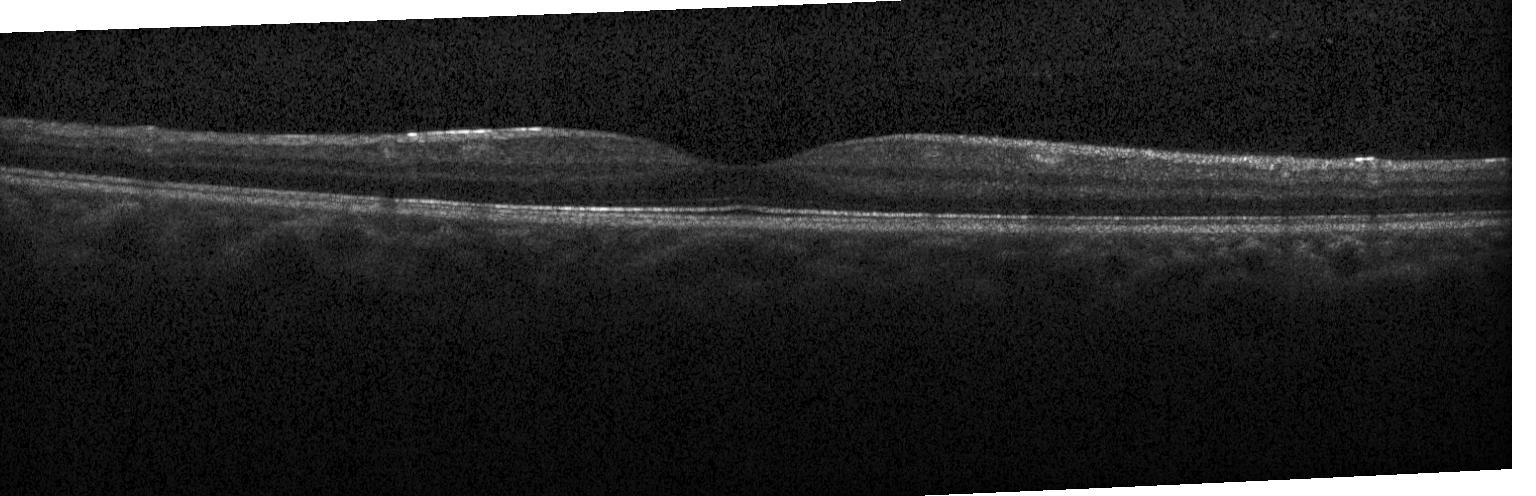
Retinal OCT cross-section showing no CNV, DME, or drusen.